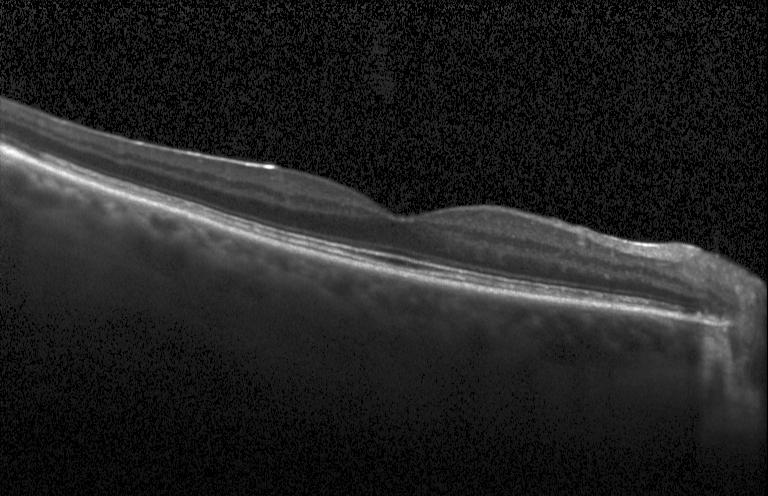
OCT B-scan · Heidelberg Spectralis · centered on the fovea — The scan shows no choroidal neovascularization, diabetic macular edema, or drusen.